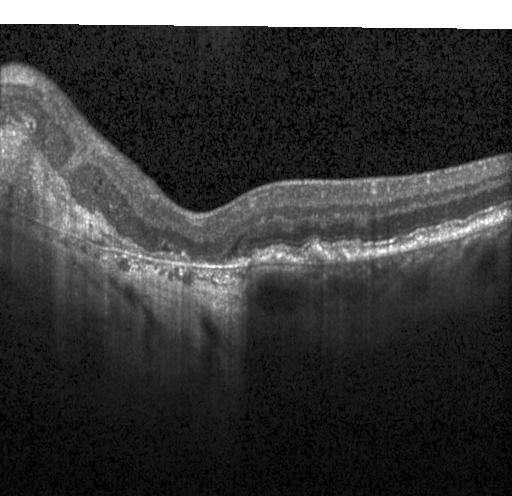 Assessment: CNV.